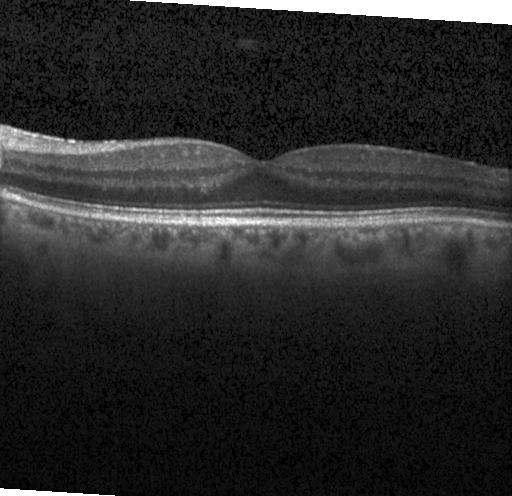

Spectral-domain optical coherence tomography. OCT line scan. Acquired on a Heidelberg Spectralis. Fovea-centered.
OCT finding: no evidence of choroidal neovascularization, diabetic macular edema, or drusen.